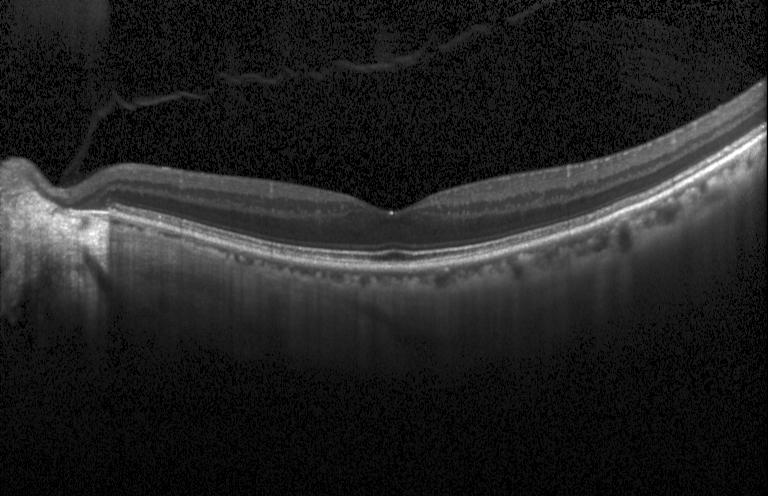 Impression: no choroidal neovascularization, no diabetic macular edema, and no drusen.